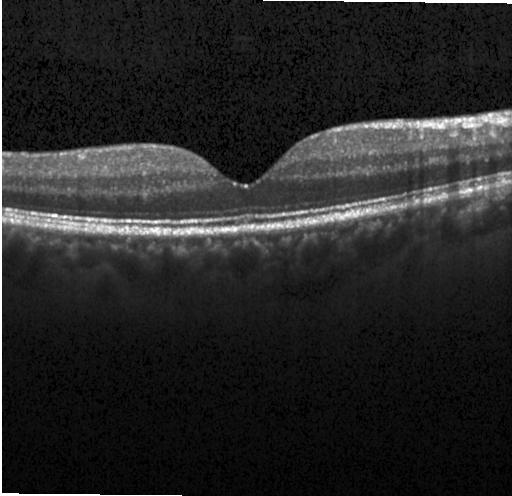
Spectral-domain OCT; optical coherence tomography B-scan.
No choroidal neovascularization, diabetic macular edema, or drusen.